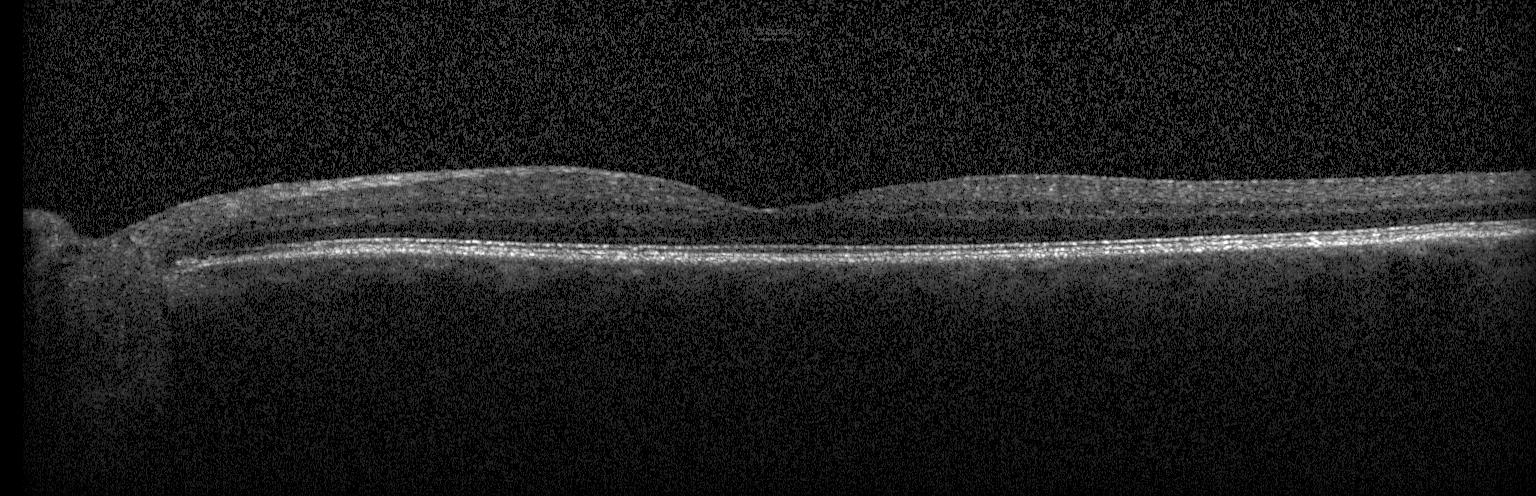

OCT finding: no CNV, DME, or drusen.